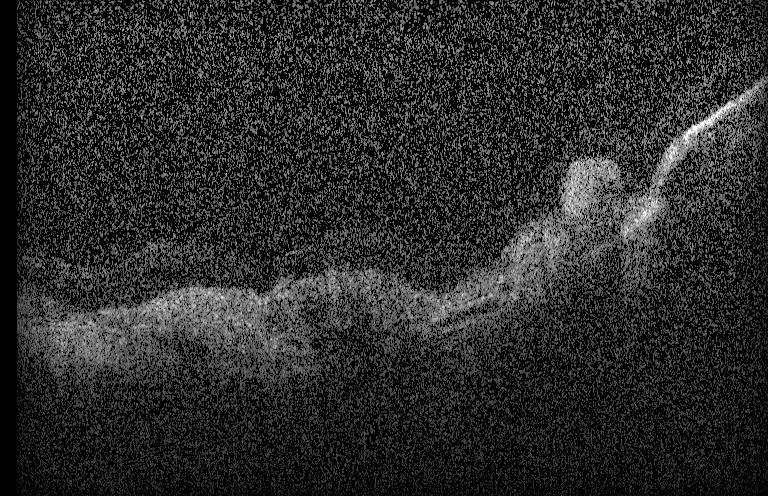
Spectral-domain OCT · Heidelberg Spectralis · macular scan · retinal OCT cross-section — Diagnosis: a choroidal neovascular membrane.